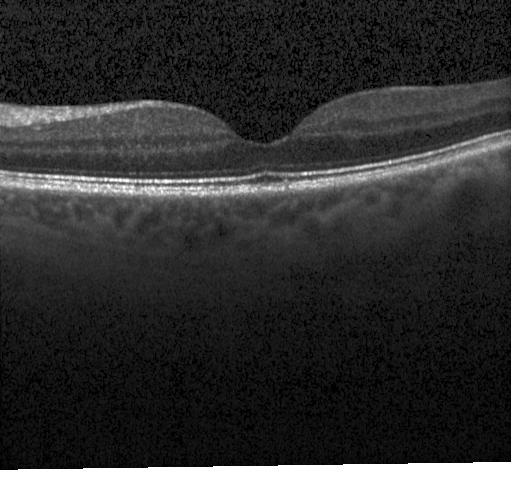 Macular OCT demonstrating no choroidal neovascularization, no diabetic macular edema, and no drusen.